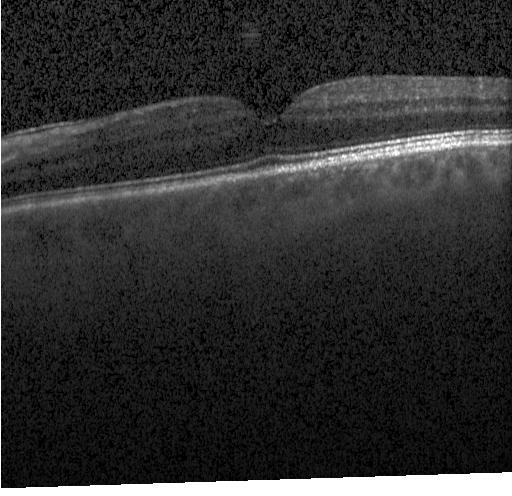

Fovea-centered · OCT B-scan
Diagnosis: neither CNV, DME, nor drusen.